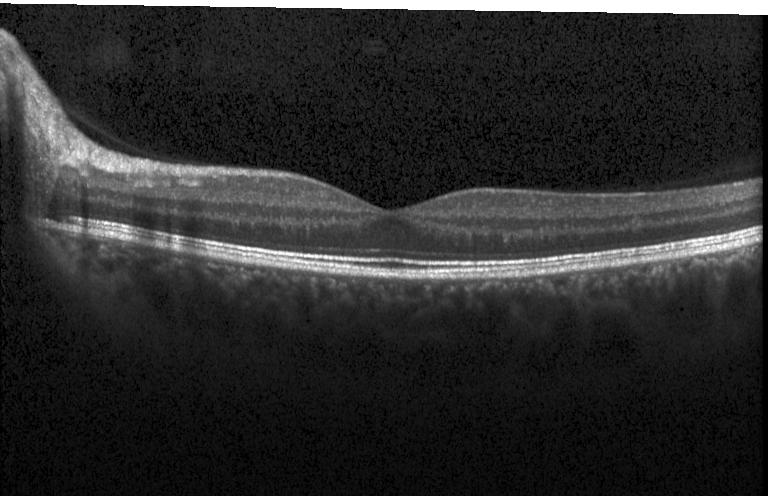
Optical coherence tomography scan. Neither CNV, DME, nor drusen.